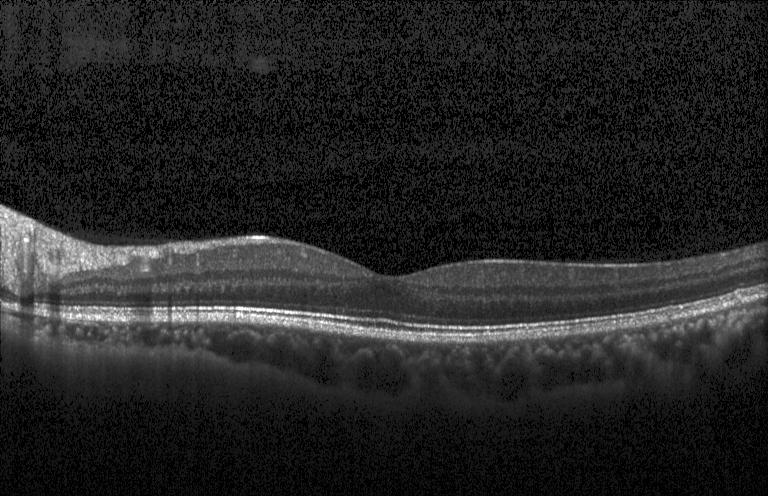
Finding: no choroidal neovascularization, no diabetic macular edema, and no drusen.